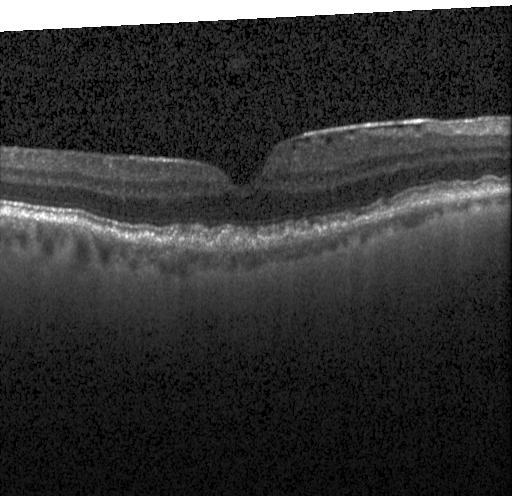 Centered on the fovea · retinal OCT cross-section — Diagnosis: sub-RPE drusenoid deposits.